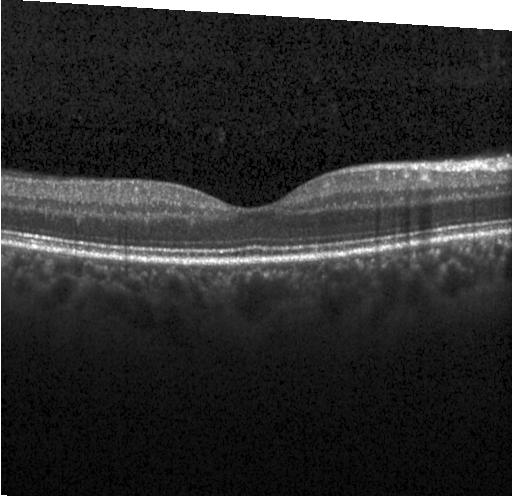 Impression: no evidence of CNV, DME, or drusen.